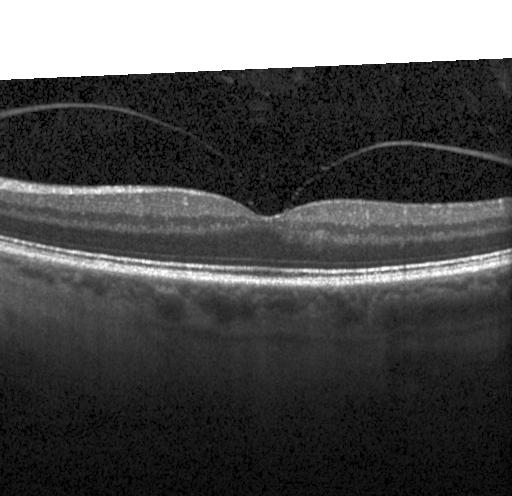 Diagnosis: no CNV, no DME, and no drusen.